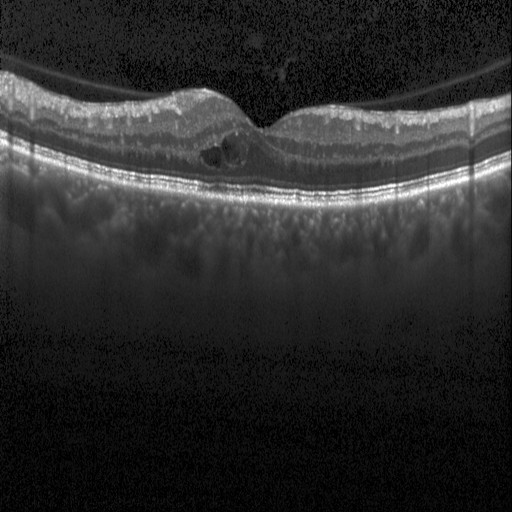

Spectral-domain optical coherence tomography. Fovea-centered. Optical coherence tomography scan
Assessment: diabetic macular edema (DME).